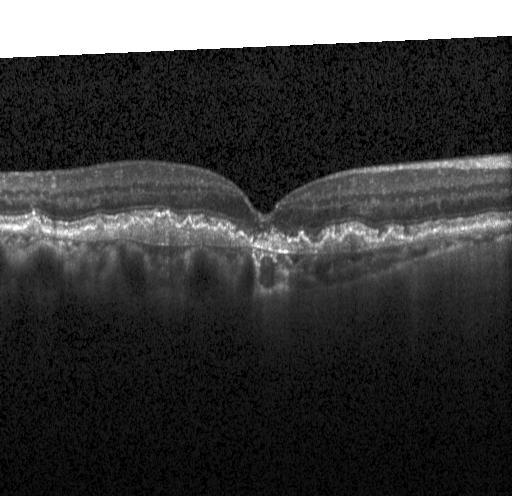

Assessment: choroidal neovascularization.